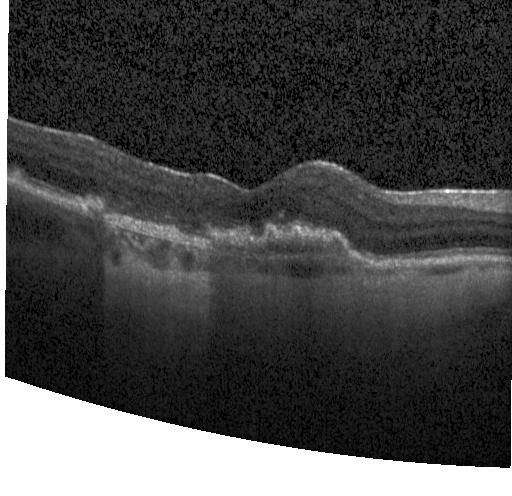 Diagnosis: a choroidal neovascular membrane.